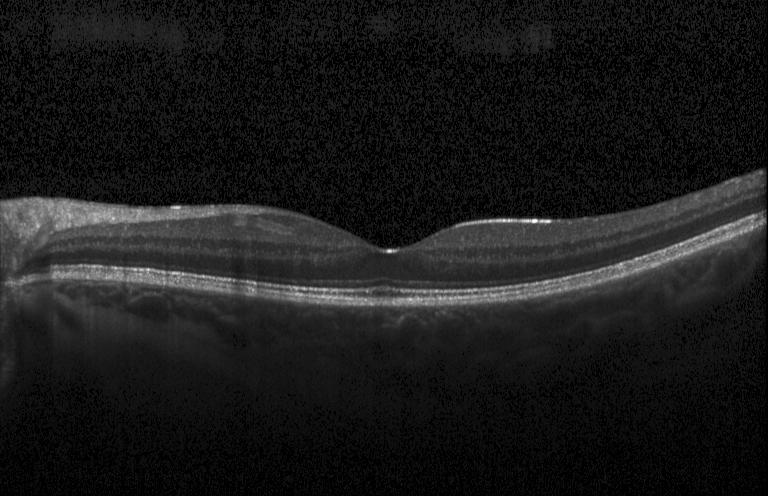
OCT B-scan · Heidelberg Spectralis OCT system
Macular OCT: neither CNV, DME, nor drusen.